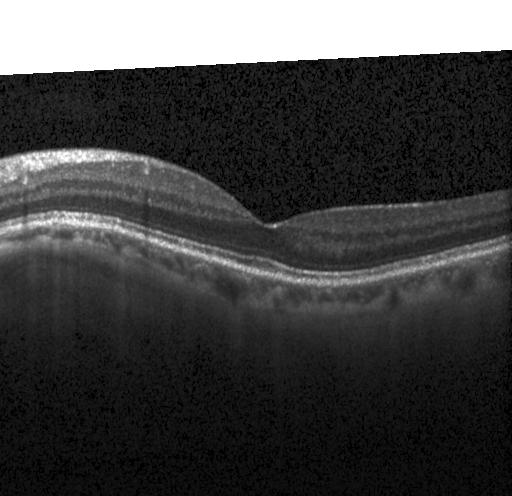

Impression: no choroidal neovascularization, diabetic macular edema, or drusen.